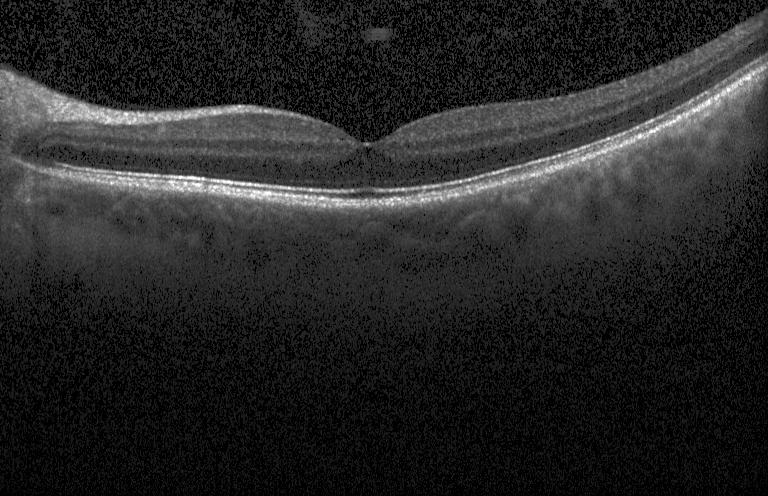 Retinal OCT cross-section. Spectral-domain optical coherence tomography. Instrument: Heidelberg Spectralis. Macular scan.
Dx: neither choroidal neovascularization, diabetic macular edema, nor drusen.